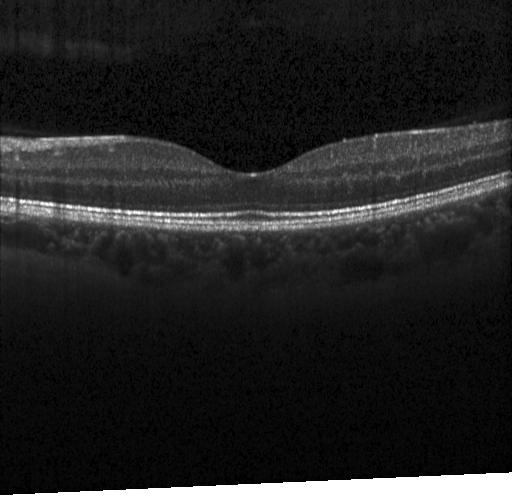

Diagnosis: neither CNV, DME, nor drusen.